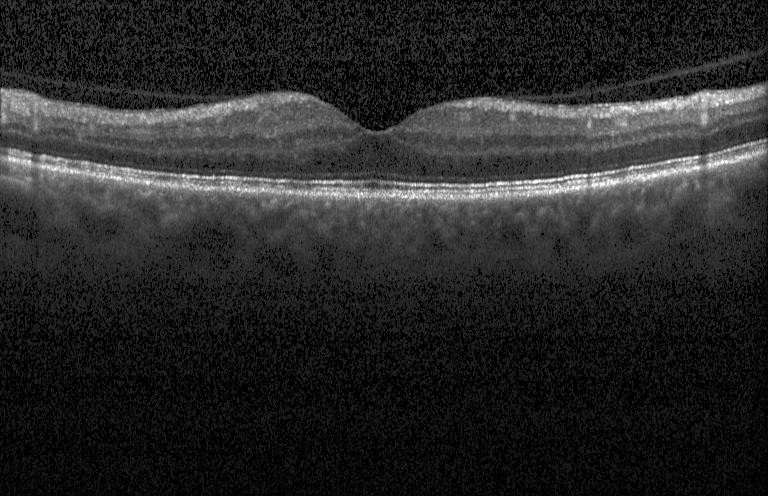 Acquired on a Heidelberg Spectralis; OCT line scan
This B-scan demonstrates no CNV, no DME, and no drusen.